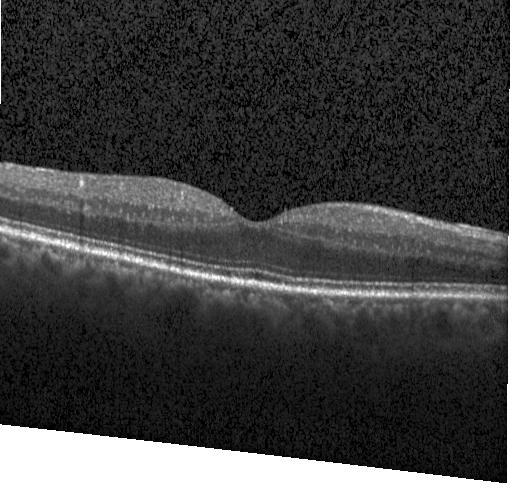

Spectral-domain optical coherence tomography. Retinal OCT B-scan. Finding: no CNV, no DME, and no drusen.